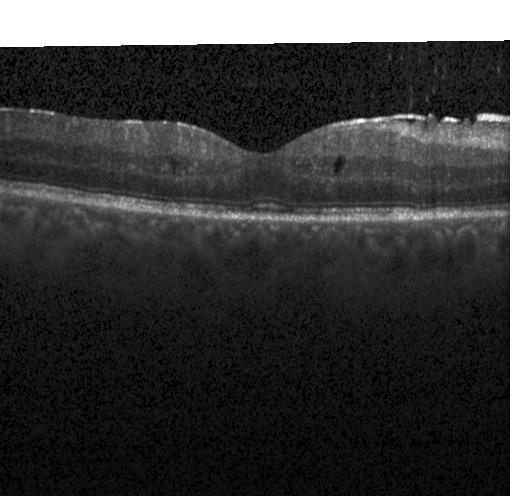 Dx: diabetic macular edema (DME).